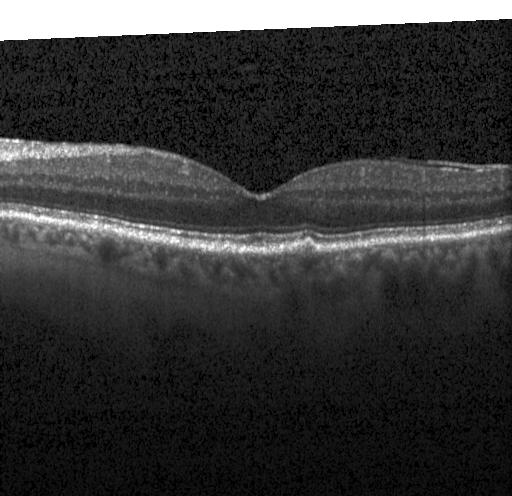 Multiple drusen.